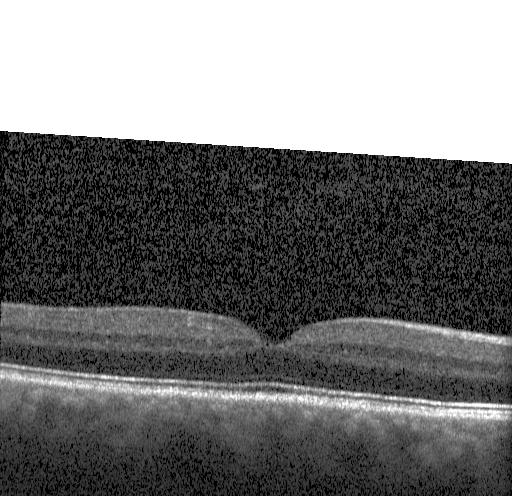 OCT line scan
This B-scan demonstrates no evidence of CNV, DME, or drusen.